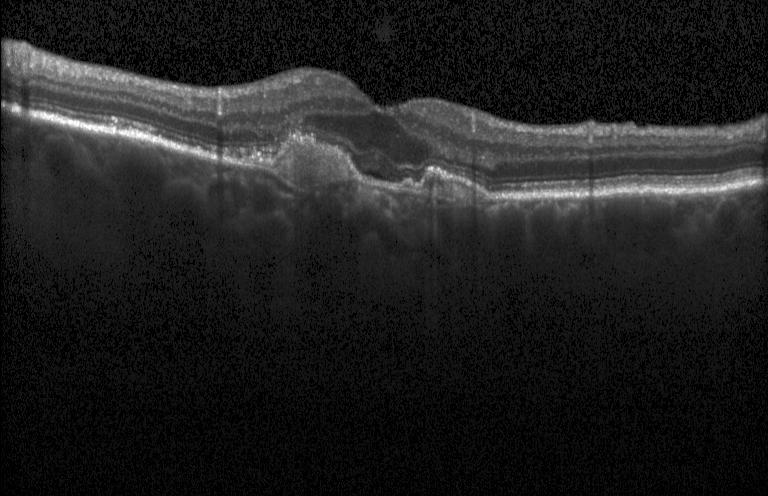 Choroidal neovascularization.